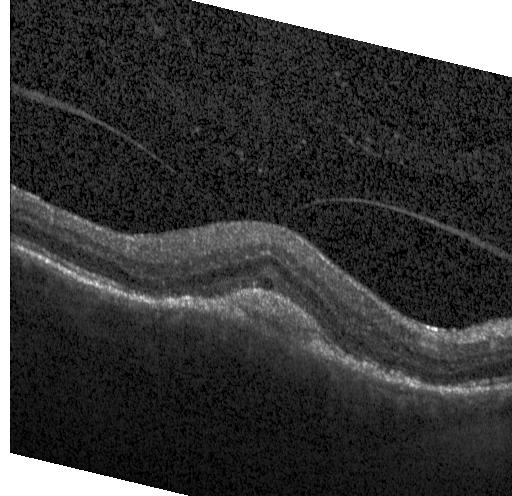 Retinal OCT cross-section showing a choroidal neovascular membrane.